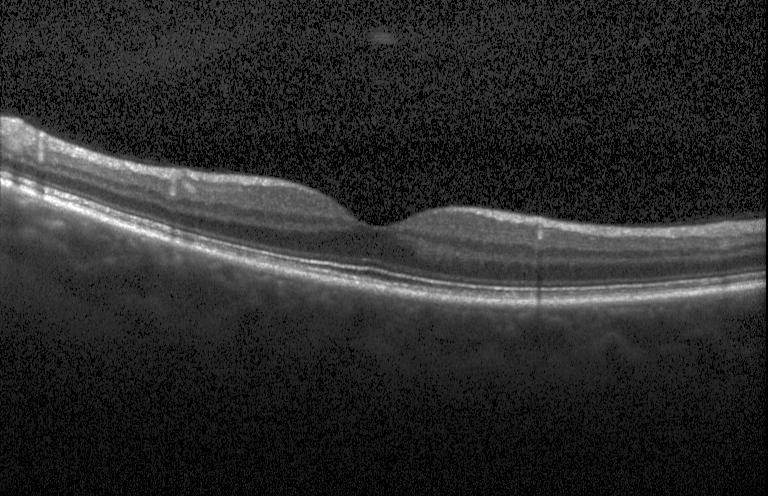
Spectral-domain optical coherence tomography. Macular scan. Optical coherence tomography scan. Instrument: Heidelberg Spectralis. OCT finding: no choroidal neovascularization, no diabetic macular edema, and no drusen.